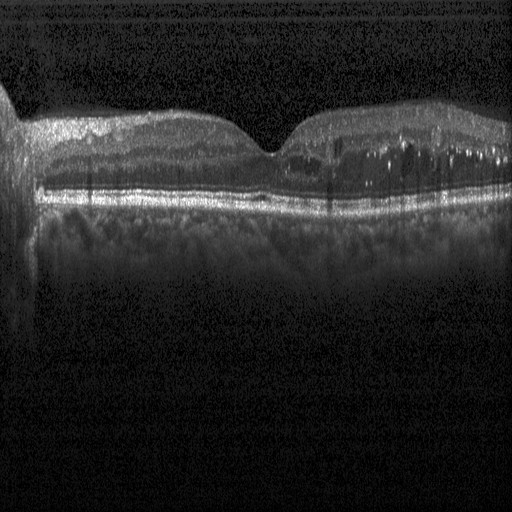 Spectral-domain OCT; macular scan; acquired on a Heidelberg Spectralis; optical coherence tomography B-scan. Impression: diabetic macular edema (DME).